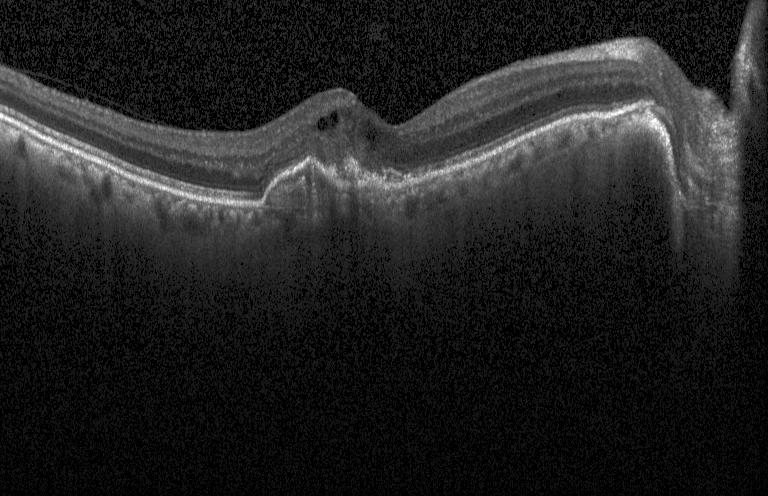 Retinal OCT B-scan, spectral-domain OCT, Heidelberg Spectralis OCT system.
Impression: a choroidal neovascular membrane.